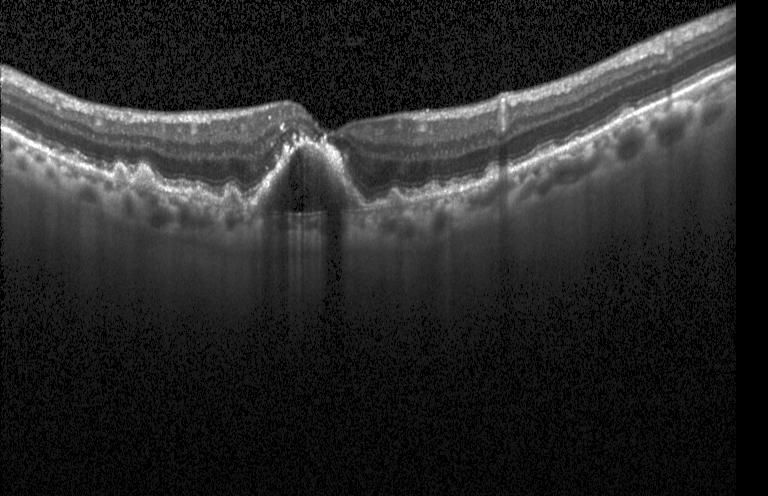

Macular OCT: choroidal neovascularization (CNV).